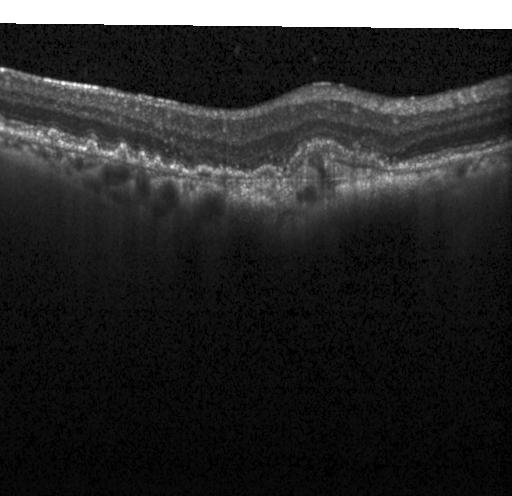
OCT B-scan showing choroidal neovascularization (CNV).